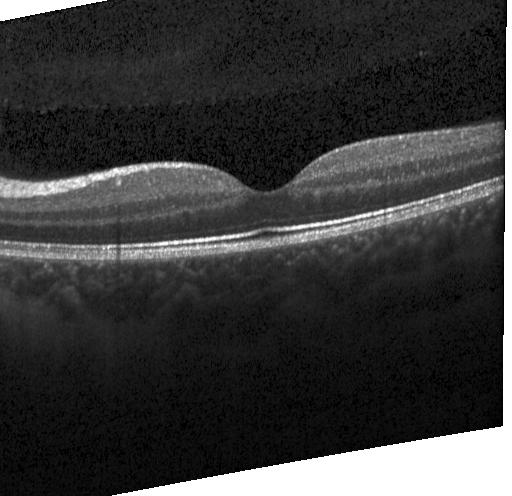
OCT B-scan. Horizontal scan through the fovea
OCT finding: no choroidal neovascularization, no diabetic macular edema, and no drusen.